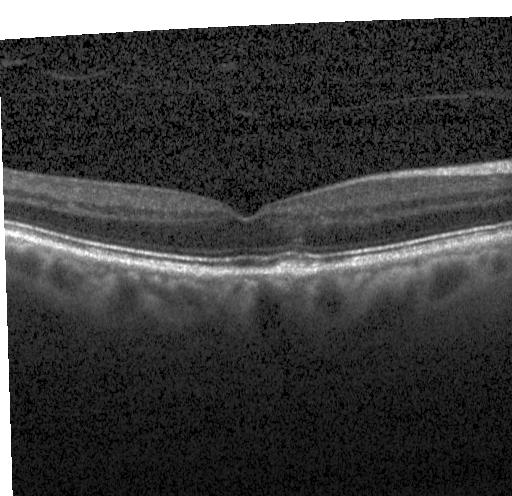 Impression: multiple drusen.